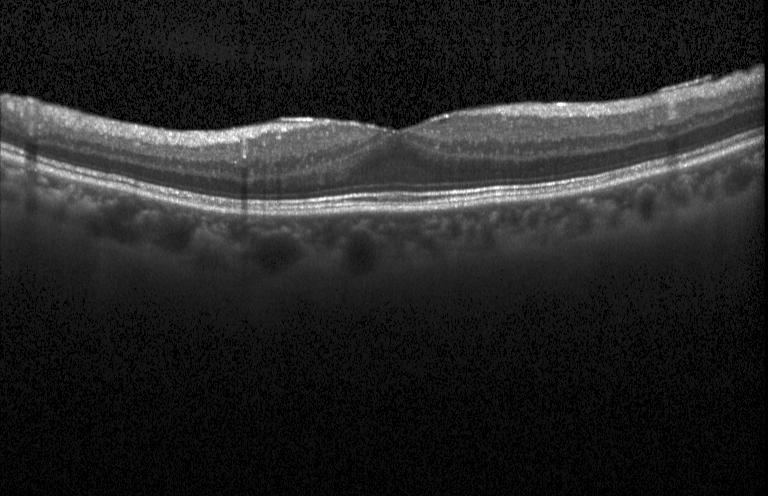 OCT B-scan · SD-OCT · fovea-centered · Heidelberg Spectralis OCT system.
Impression: no choroidal neovascularization, no diabetic macular edema, and no drusen.